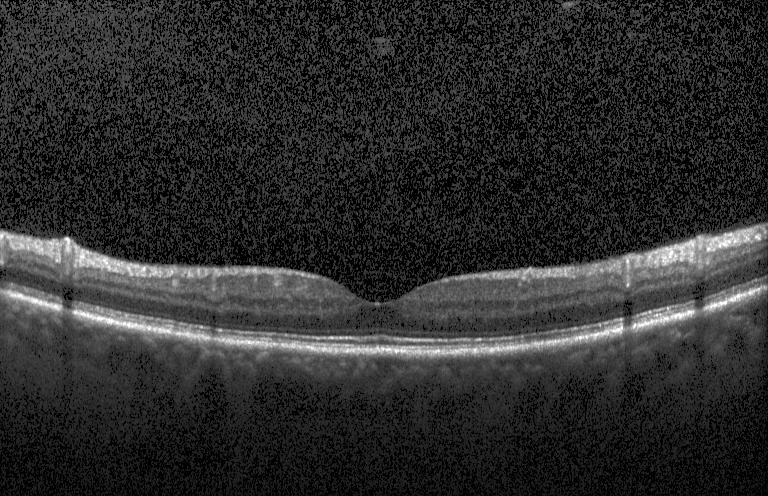 Optical coherence tomography B-scan, SD-OCT, instrument: Heidelberg Spectralis, macular scan — The scan shows no CNV, no DME, and no drusen.